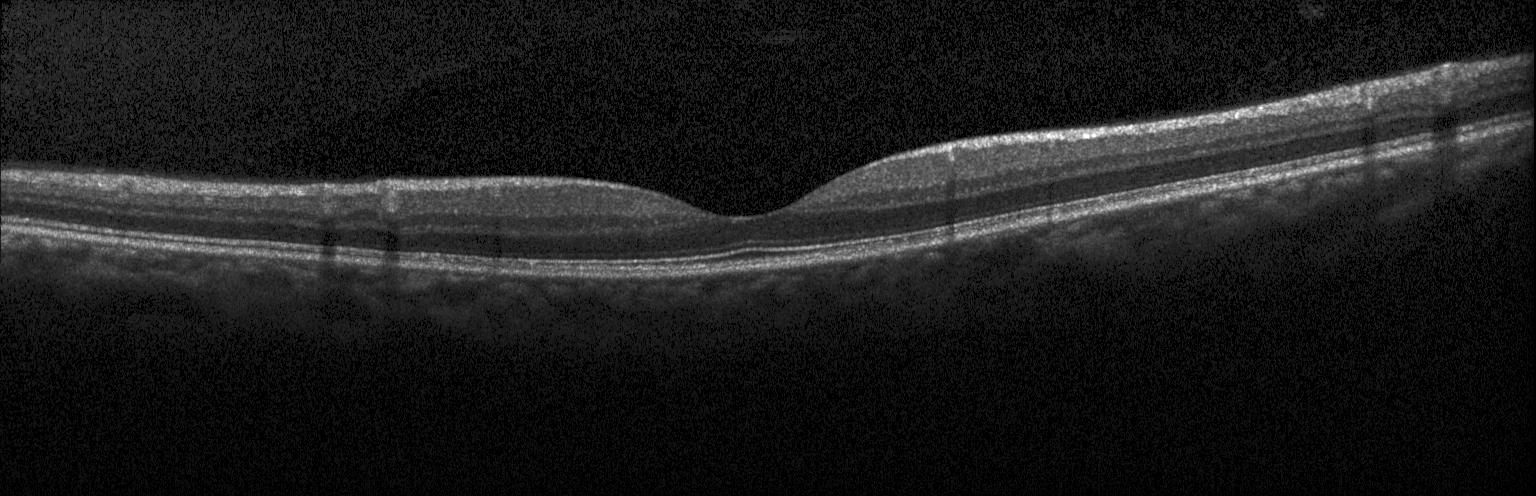

No evidence of choroidal neovascularization, diabetic macular edema, or drusen.